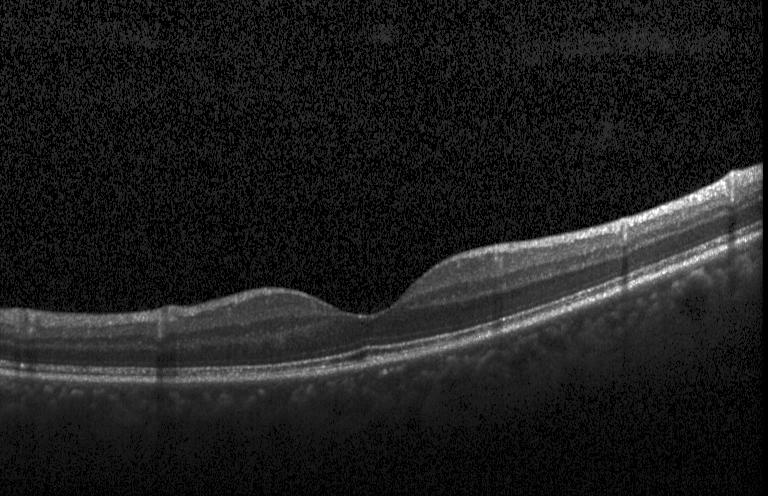

OCT finding: no CNV, no DME, and no drusen.